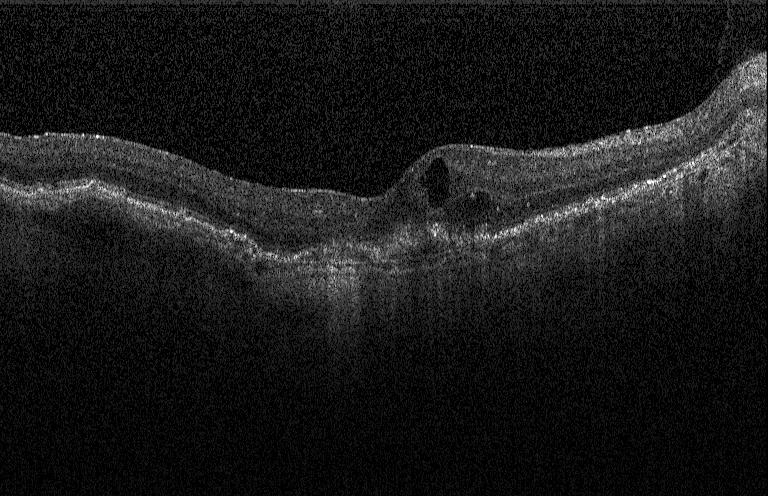
OCT line scan.
Diagnosis: choroidal neovascularization.